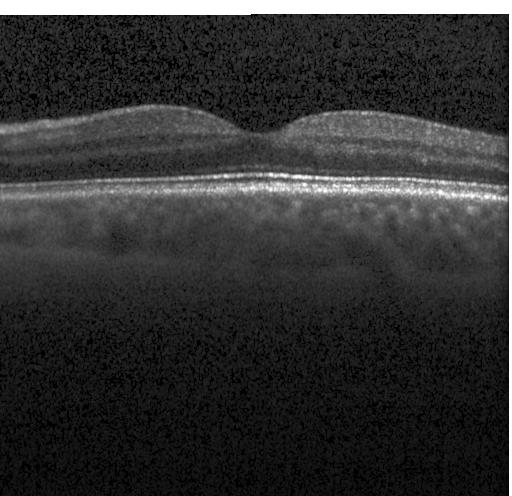 Finding: no CNV, no DME, and no drusen.